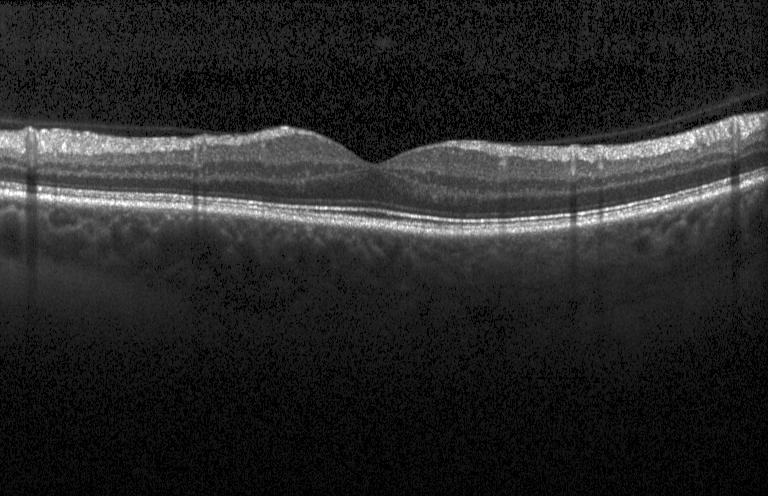

Spectral-domain OCT B-scan: neither CNV, DME, nor drusen.